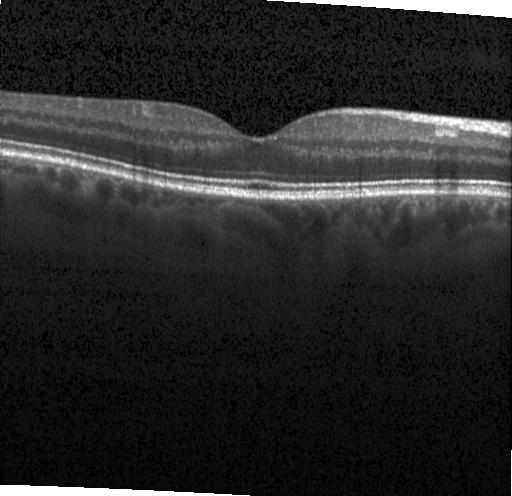
Macular scan; Heidelberg Spectralis OCT system; retinal OCT cross-section — Diagnosis: no choroidal neovascularization, no diabetic macular edema, and no drusen.